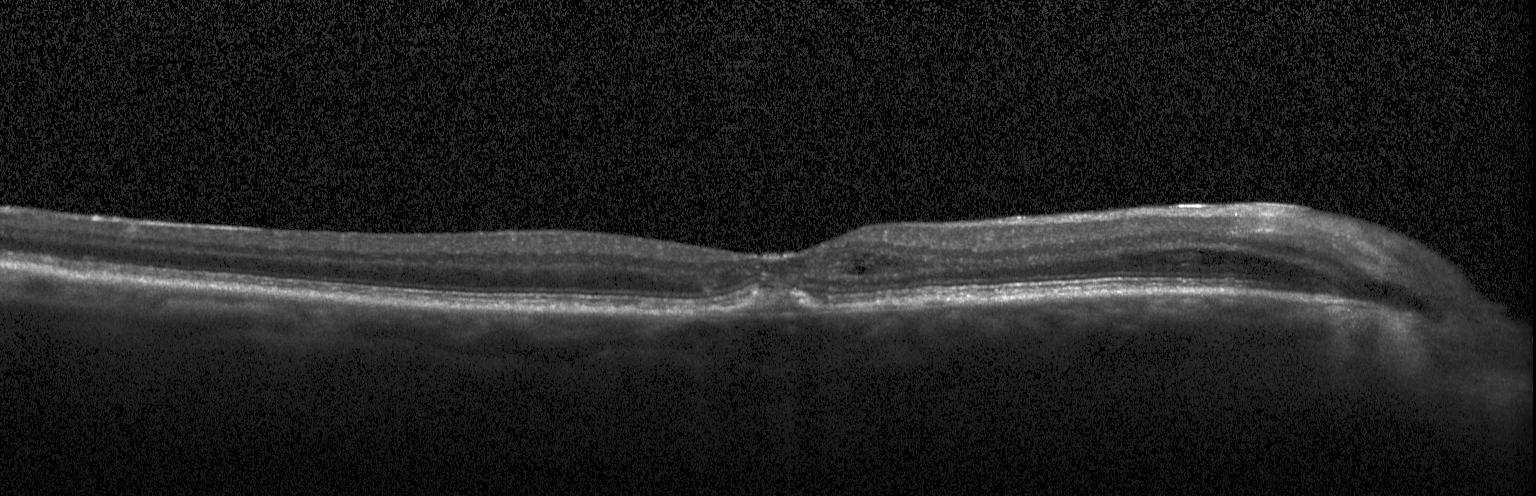 OCT finding: choroidal neovascularization.